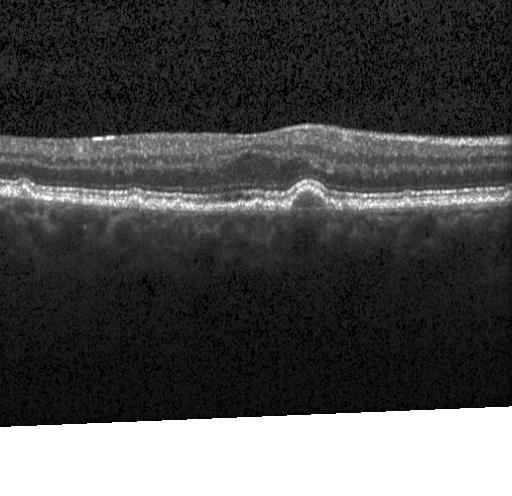

Finding: sub-RPE drusenoid deposits.